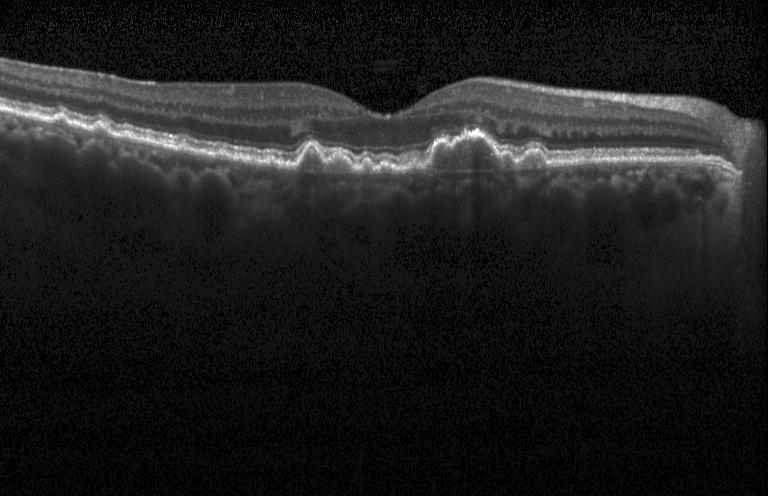
Assessment: drusen.